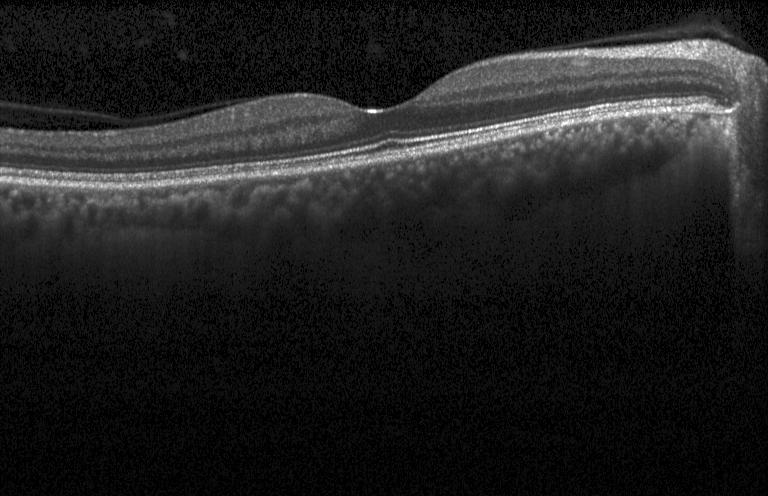

Finding: no CNV, no DME, and no drusen.